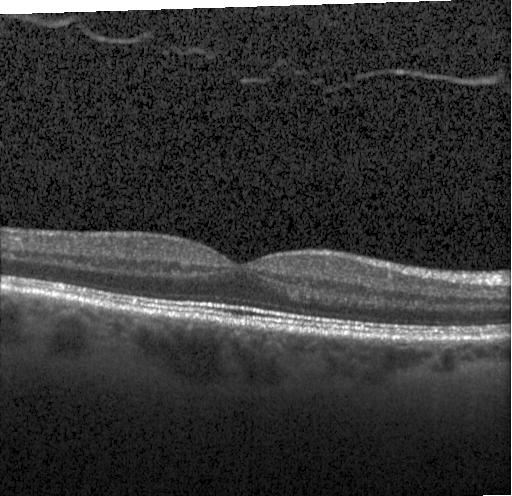
Horizontal scan through the fovea · instrument: Heidelberg Spectralis · optical coherence tomography B-scan.
No choroidal neovascularization, diabetic macular edema, or drusen.